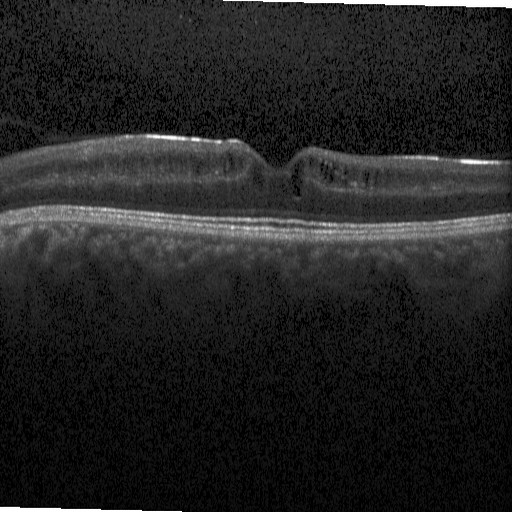 OCT B-scan; centered on the fovea.
Assessment: diabetic macular edema.